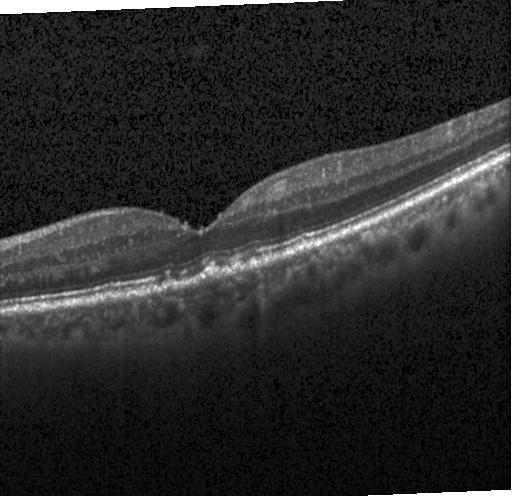

Impression: multiple drusen.